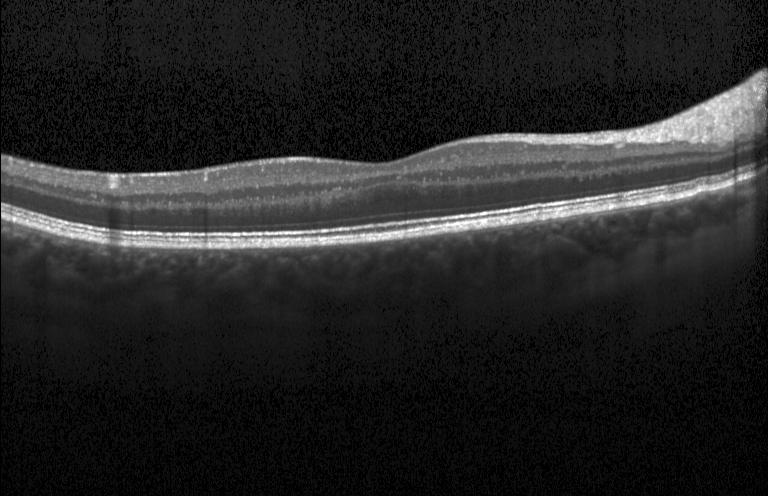

OCT B-scan showing no CNV, DME, or drusen.